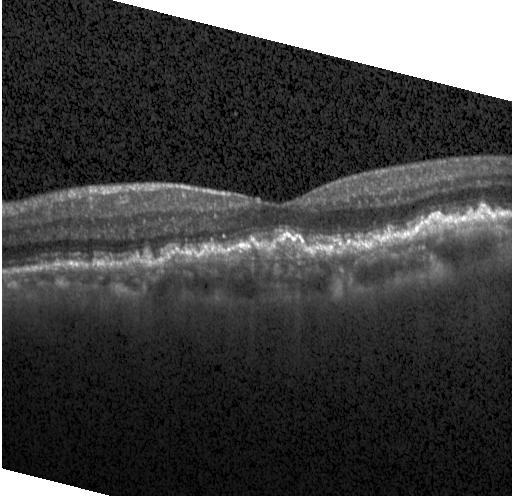 Centered on the fovea, retinal OCT B-scan, acquired on a Heidelberg Spectralis, spectral-domain optical coherence tomography.
Macular OCT: choroidal neovascularization (CNV).